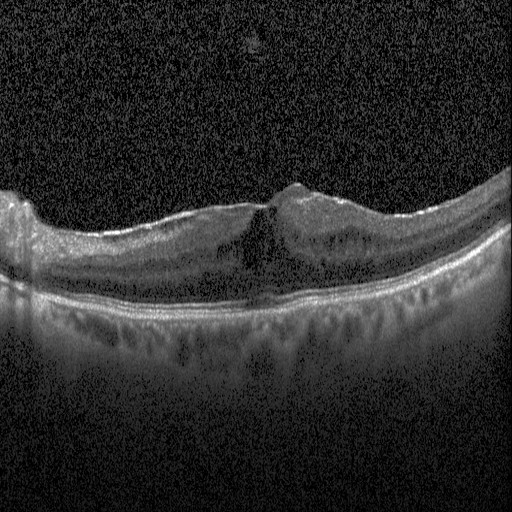
Diabetic macular edema (DME).